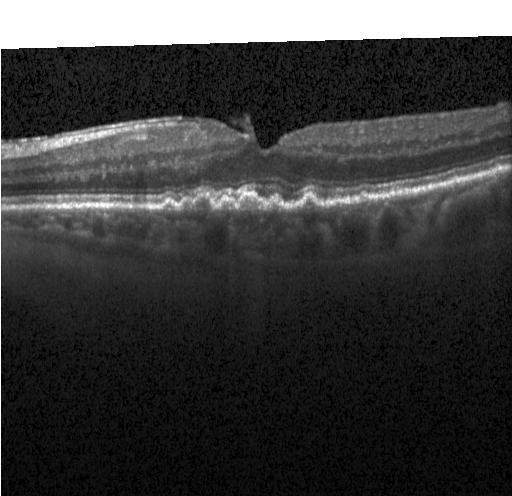 Macular OCT demonstrating sub-RPE drusenoid deposits.